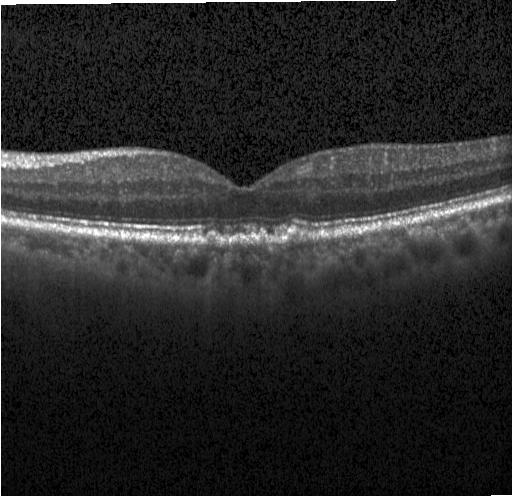

Spectral-domain OCT · horizontal scan through the fovea · optical coherence tomography B-scan
Diagnosis: sub-RPE drusenoid deposits.